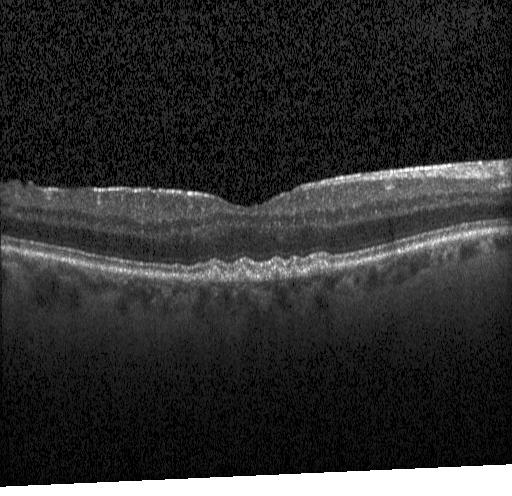 Impression: multiple drusen.